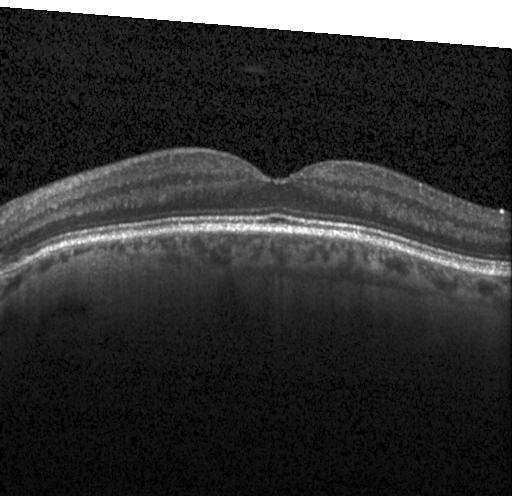
OCT B-scan. Diagnosis: no evidence of CNV, DME, or drusen.